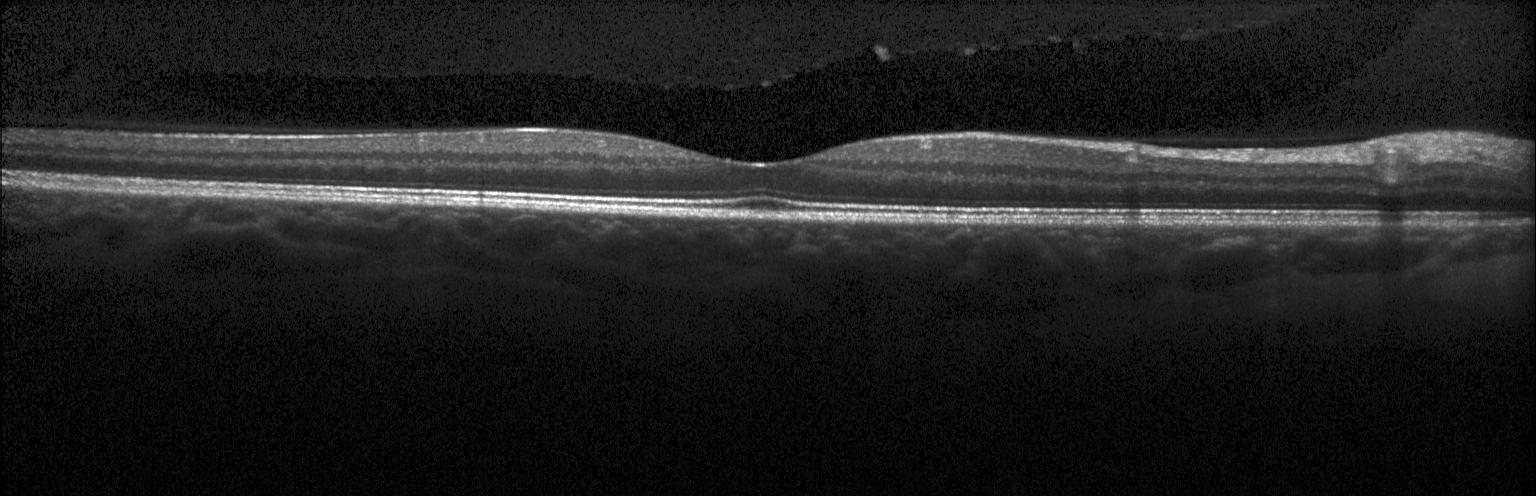 No choroidal neovascularization, no diabetic macular edema, and no drusen.